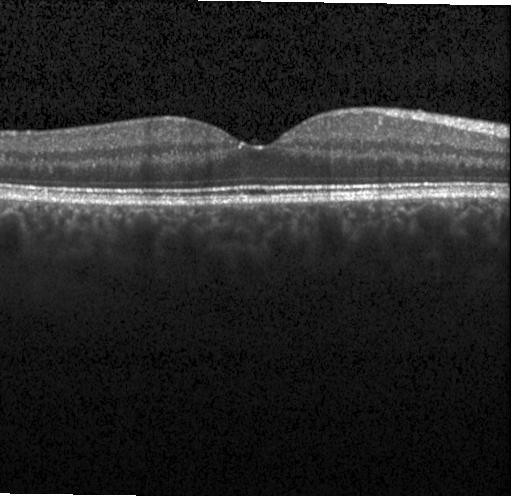
Optical coherence tomography scan. Heidelberg Spectralis. Fovea-centered. SD-OCT — Impression: no CNV, no DME, and no drusen.